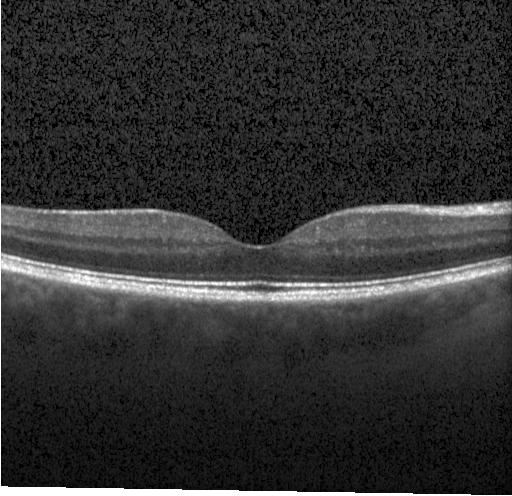 Retinal OCT B-scan; acquired on a Heidelberg Spectralis; centered on the fovea.
Dx: neither CNV, DME, nor drusen.